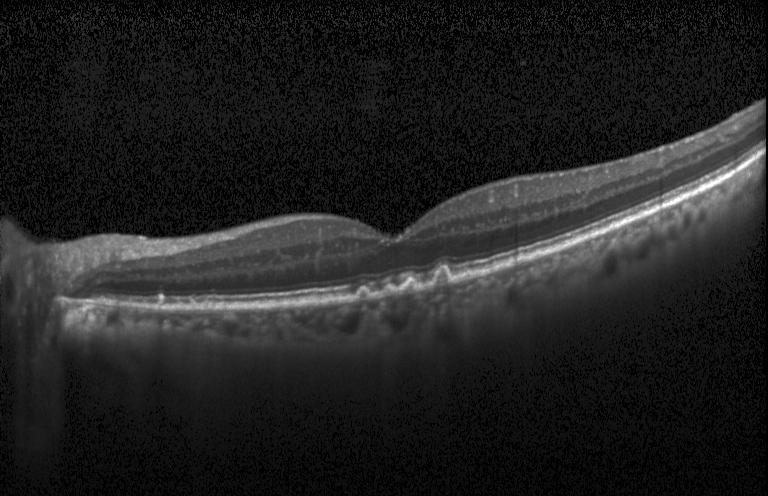 SD-OCT · optical coherence tomography scan. Diagnosis: multiple drusen.